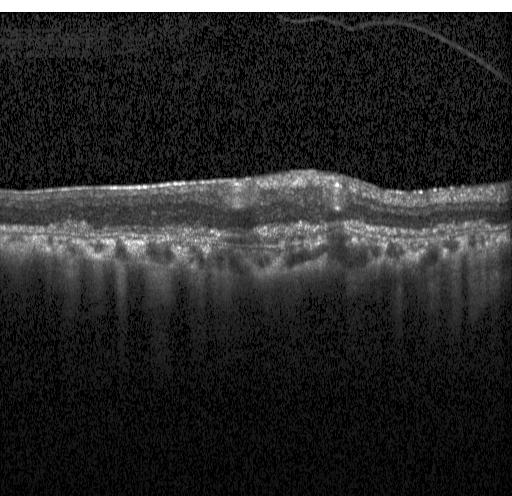

Spectral-domain OCT B-scan: choroidal neovascularization.